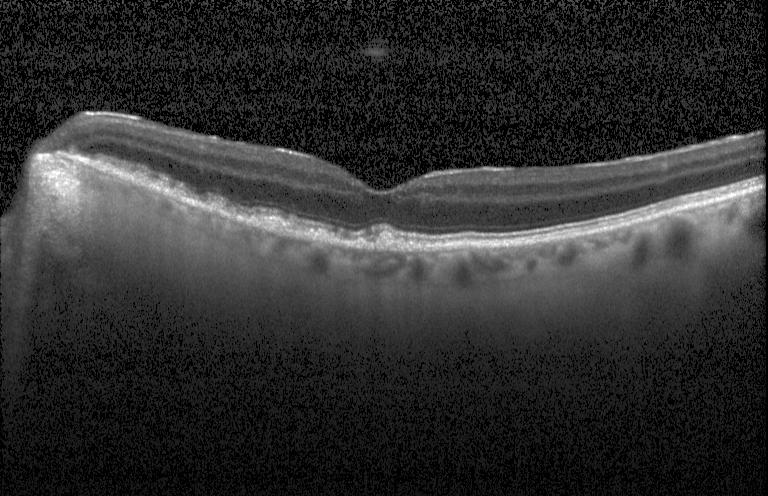 Instrument: Heidelberg Spectralis; optical coherence tomography B-scan — OCT finding: drusen.